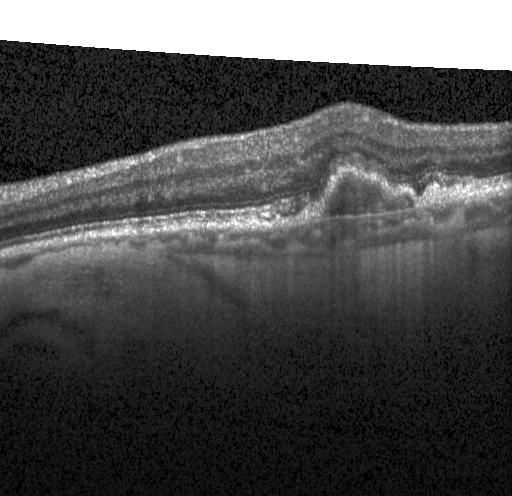
Retinal OCT cross-section
Finding: choroidal neovascularization.